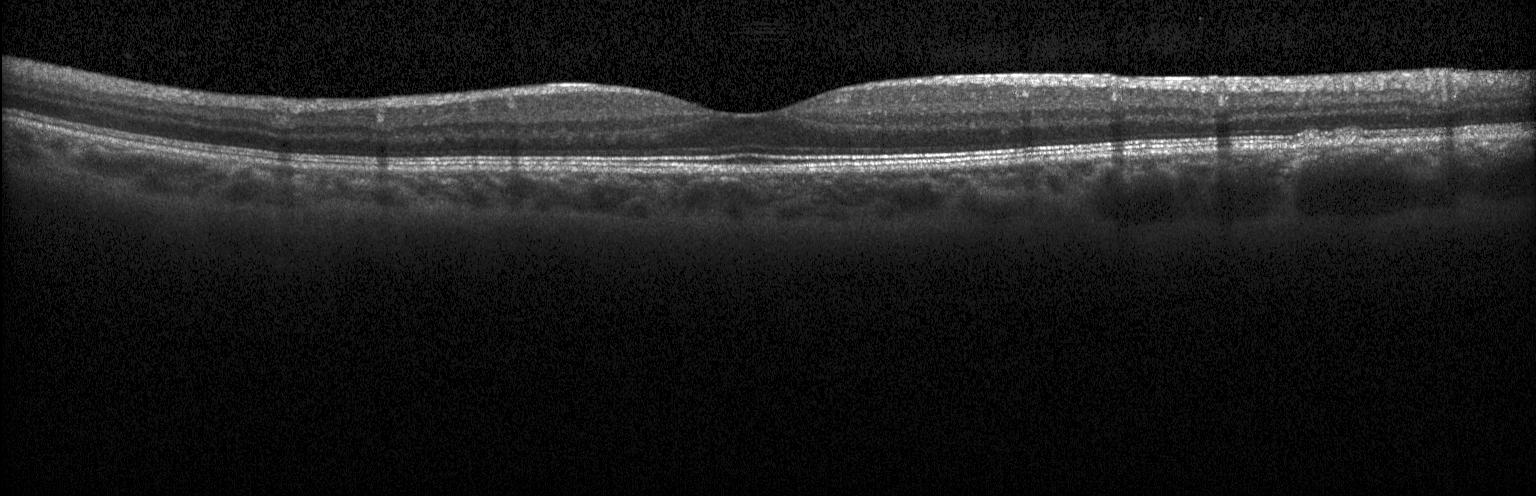 OCT finding: drusen.